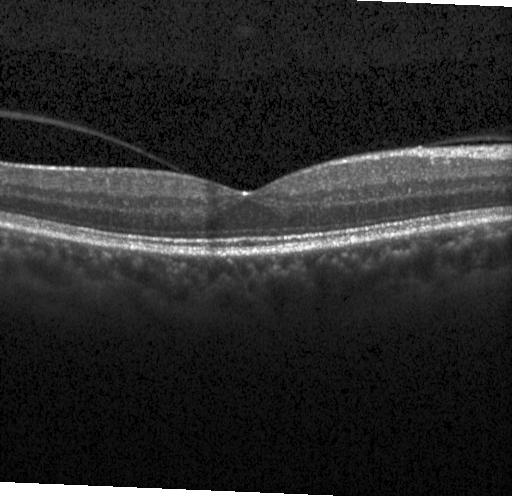

Diagnosis: no evidence of CNV, DME, or drusen.